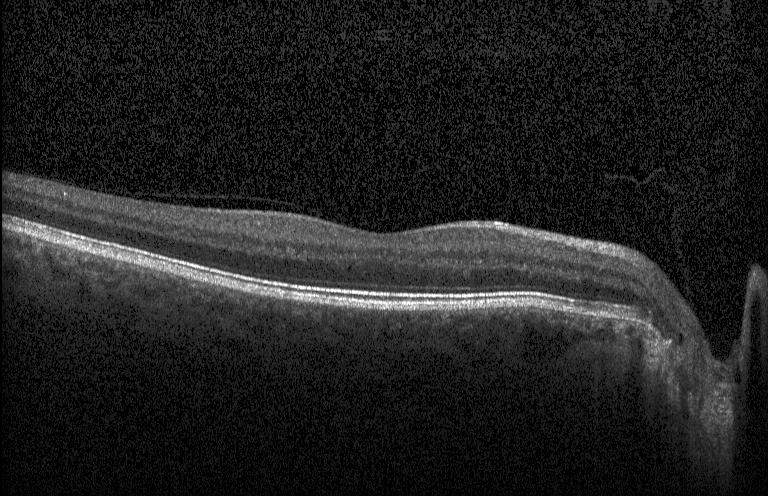 Diagnosis: no evidence of CNV, DME, or drusen.